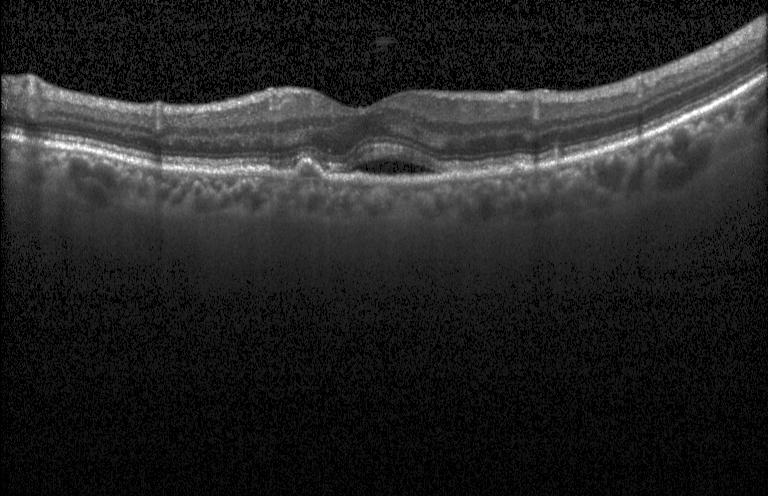 OCT line scan — This B-scan demonstrates a choroidal neovascular membrane.